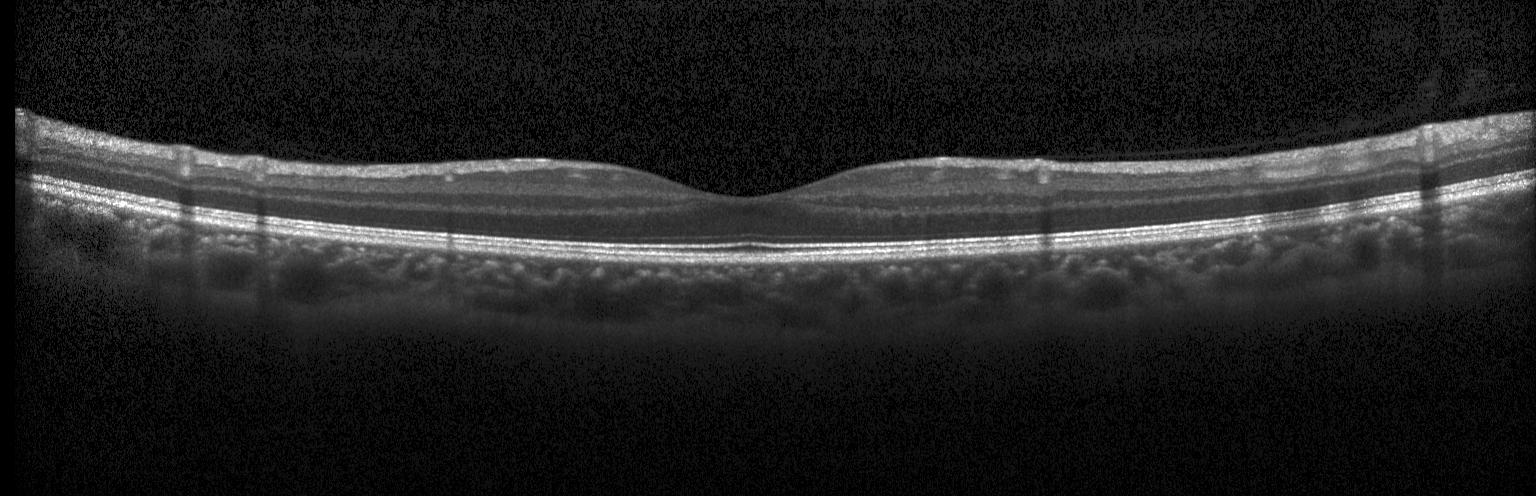

Macular scan, SD-OCT, Heidelberg Spectralis OCT system, optical coherence tomography scan — Diagnosis: no choroidal neovascularization, diabetic macular edema, or drusen.